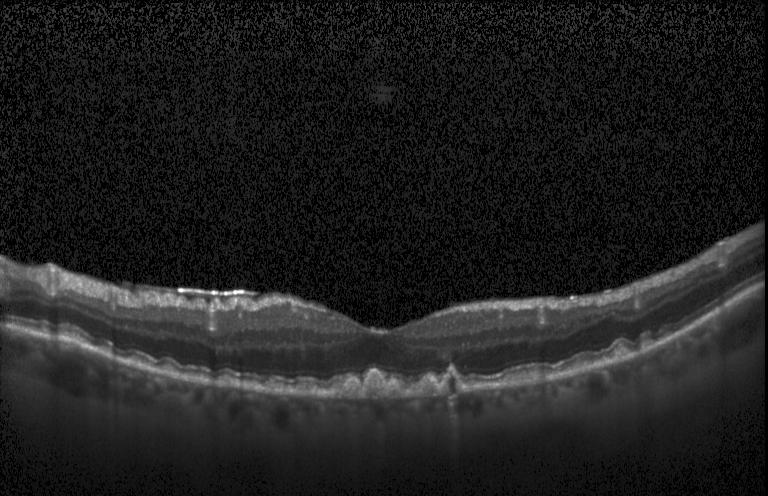 Optical coherence tomography B-scan.
Sub-RPE drusenoid deposits.